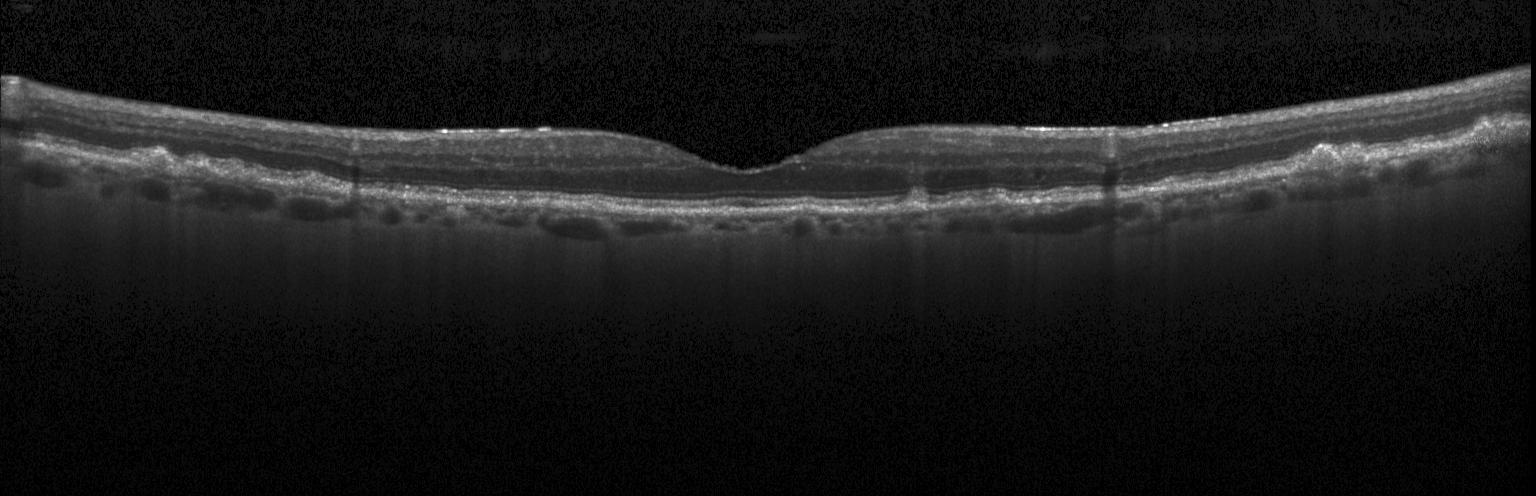 Retinal OCT cross-section. Multiple drusen.